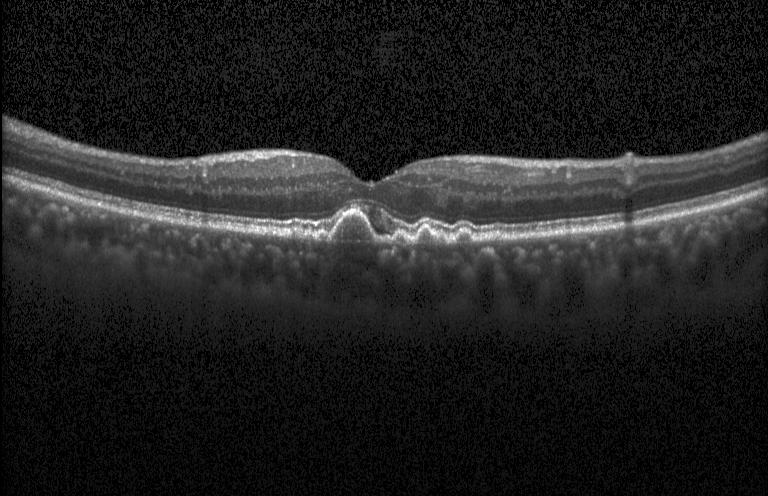 Instrument: Heidelberg Spectralis. Retinal OCT cross-section. Horizontal scan through the fovea
Finding: drusen.